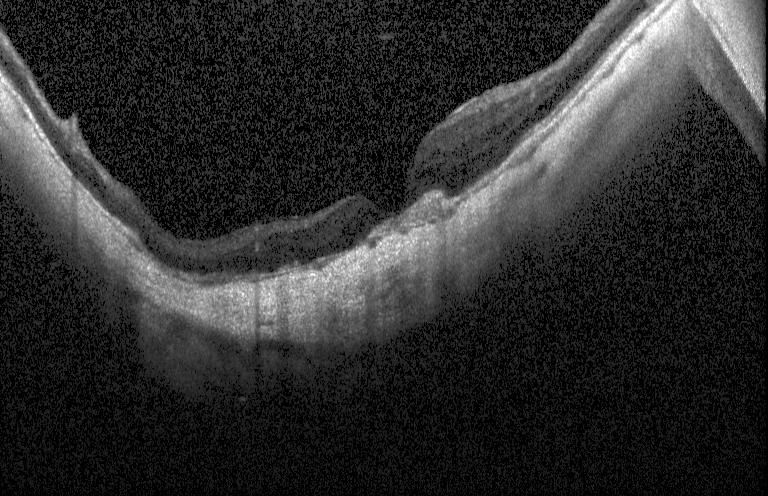 OCT B-scan. Centered on the fovea. Instrument: Heidelberg Spectralis. This B-scan demonstrates a choroidal neovascular membrane.